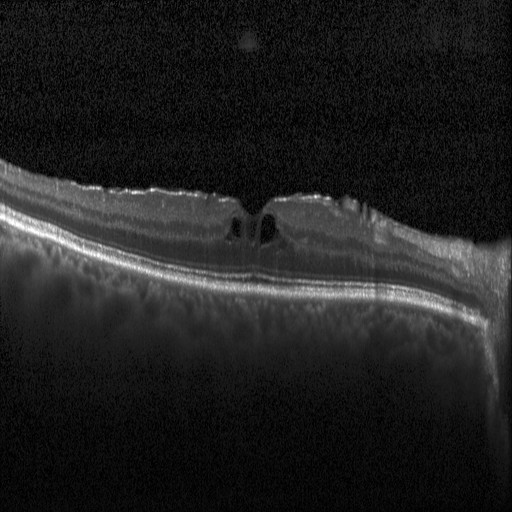
Retinal OCT B-scan, centered on the fovea — Assessment: diabetic macular edema (DME).